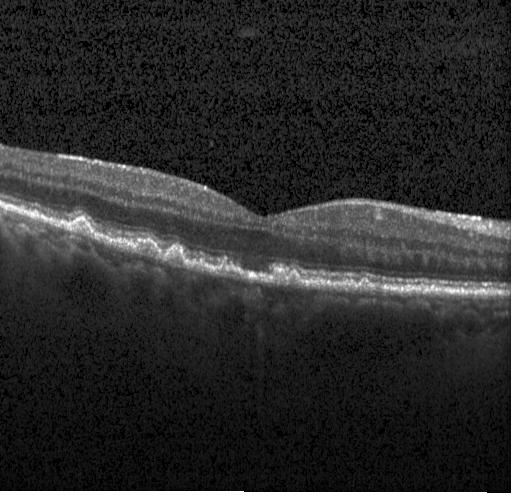

Macular OCT: multiple drusen.